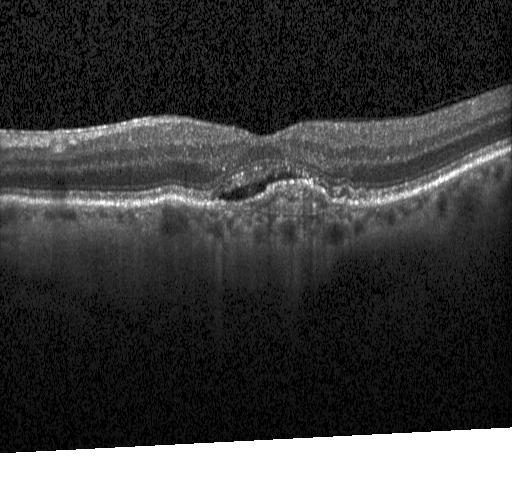

Instrument: Heidelberg Spectralis; centered on the fovea; spectral-domain OCT; optical coherence tomography scan
Diagnosis: choroidal neovascularization (CNV).